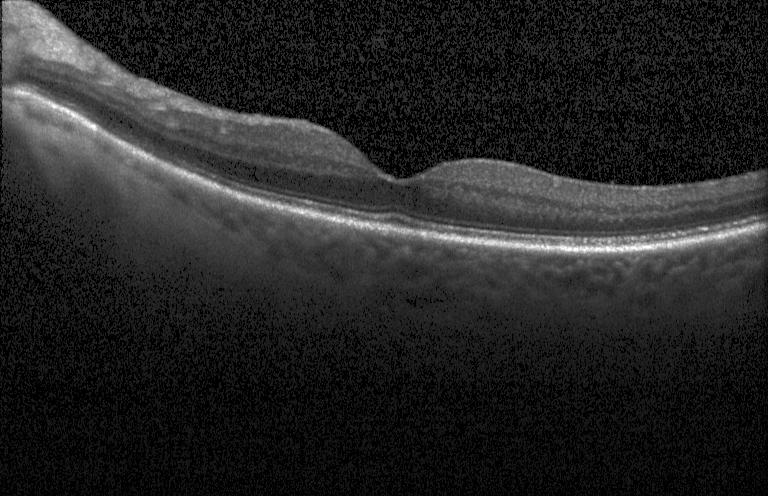
Heidelberg Spectralis OCT system, macular scan, retinal OCT B-scan, SD-OCT.
Diagnosis: no evidence of CNV, DME, or drusen.